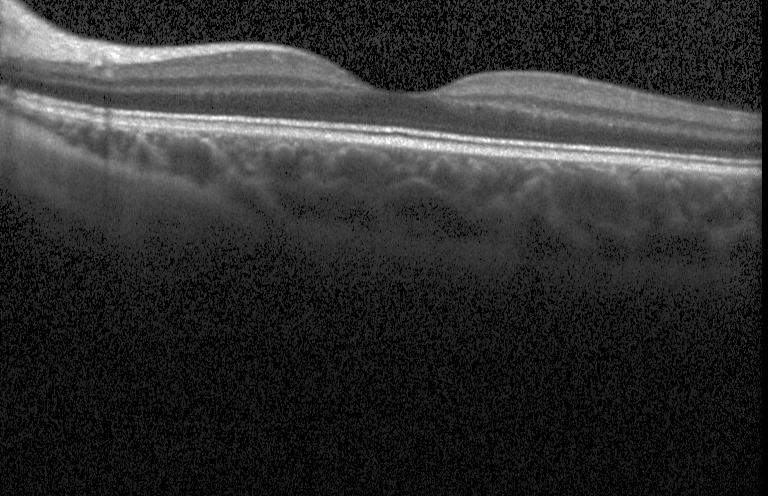
Through the macula. SD-OCT. OCT B-scan. Finding: neither choroidal neovascularization, diabetic macular edema, nor drusen.